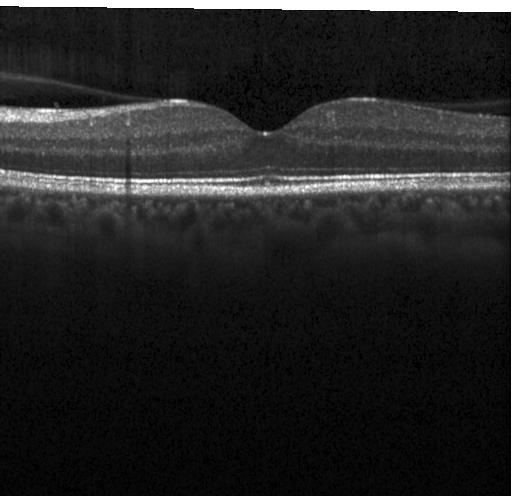 This B-scan demonstrates no choroidal neovascularization, no diabetic macular edema, and no drusen.